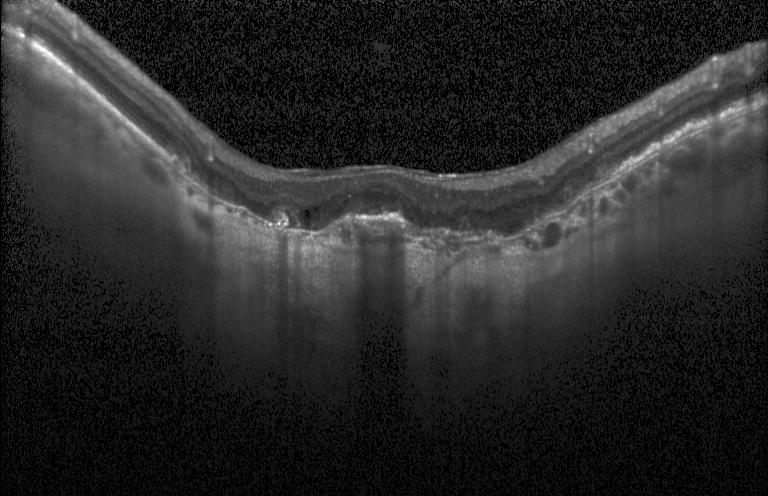
SD-OCT; macular scan; optical coherence tomography scan. Diagnosis: a choroidal neovascular membrane.